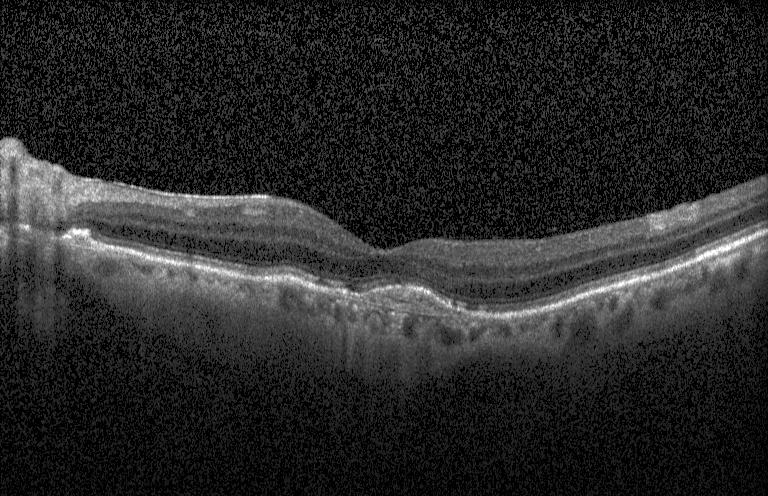

Optical coherence tomography B-scan.
Finding: a choroidal neovascular membrane.